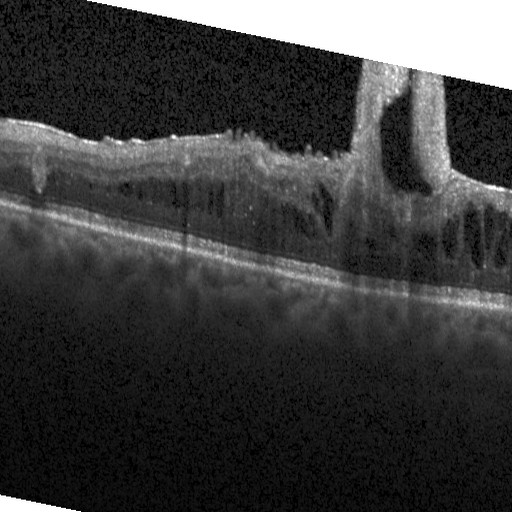
OCT B-scan — Finding: diabetic macular edema (DME).